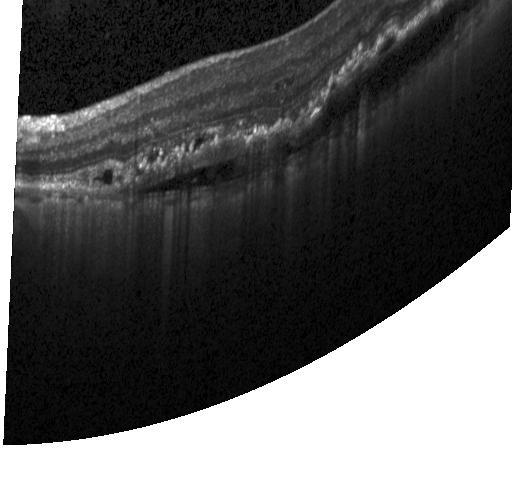 OCT line scan. Impression: choroidal neovascularization.